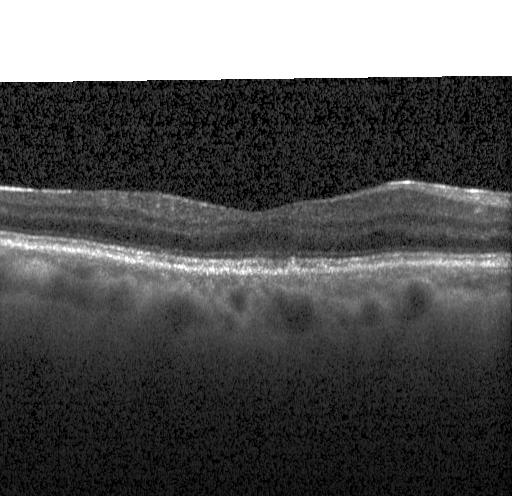

OCT B-scan. OCT finding: sub-RPE drusenoid deposits.